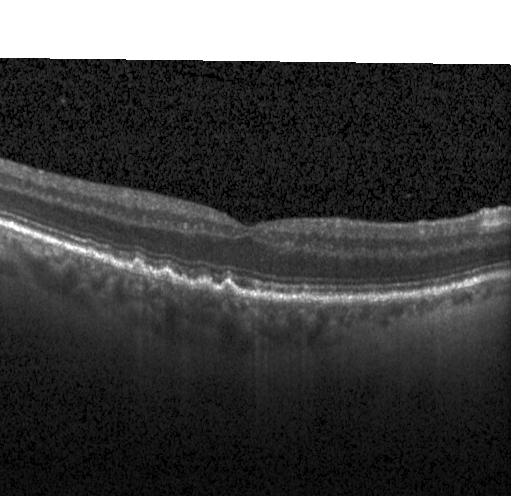

Retinal OCT cross-section showing multiple drusen.